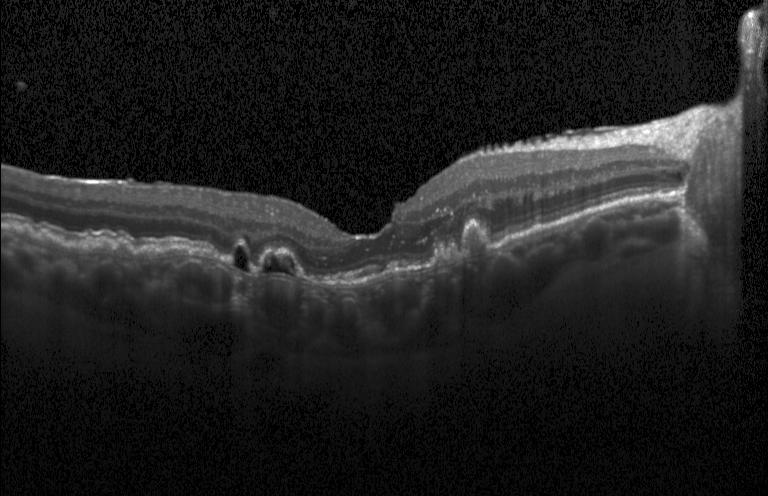 Centered on the fovea; SD-OCT; Heidelberg Spectralis; OCT line scan.
Assessment: CNV.